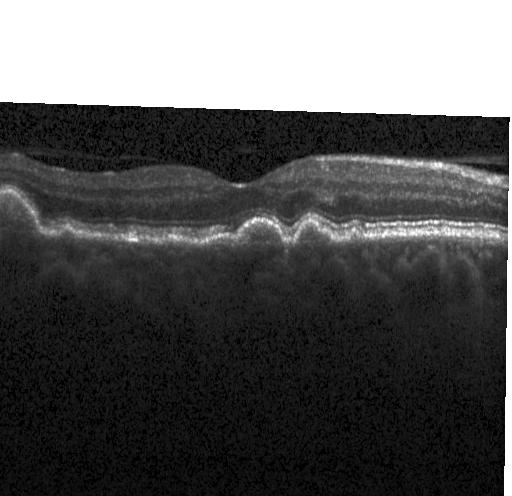
Optical coherence tomography scan. SD-OCT
This B-scan demonstrates drusen.